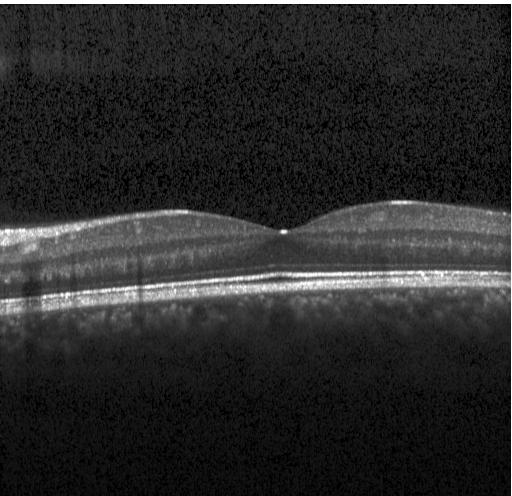

Horizontal scan through the fovea · optical coherence tomography B-scan. Macular OCT: no choroidal neovascularization, no diabetic macular edema, and no drusen.